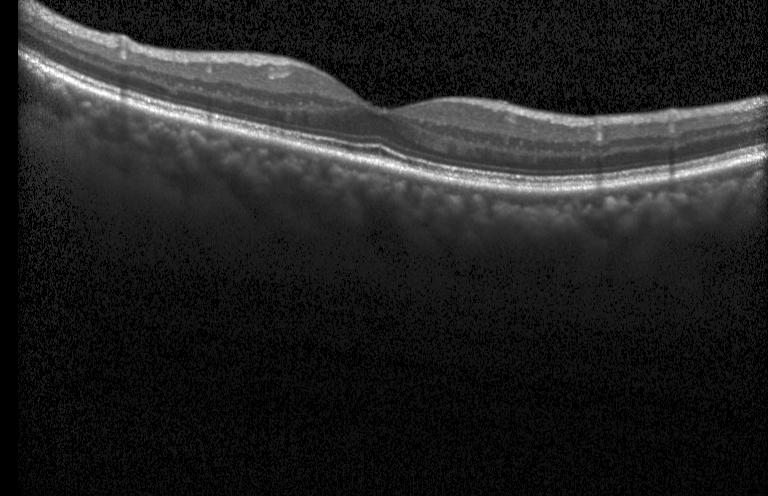
Retinal OCT B-scan, instrument: Heidelberg Spectralis, spectral-domain optical coherence tomography, macular scan. Finding: no choroidal neovascularization, no diabetic macular edema, and no drusen.